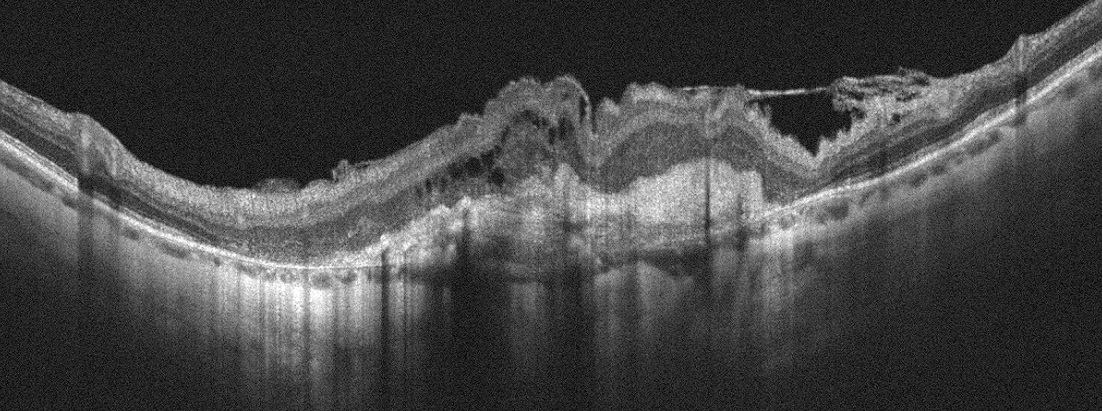

Retinal OCT B-scan · through the macula.
Macular OCT: age-related macular degeneration (AMD).